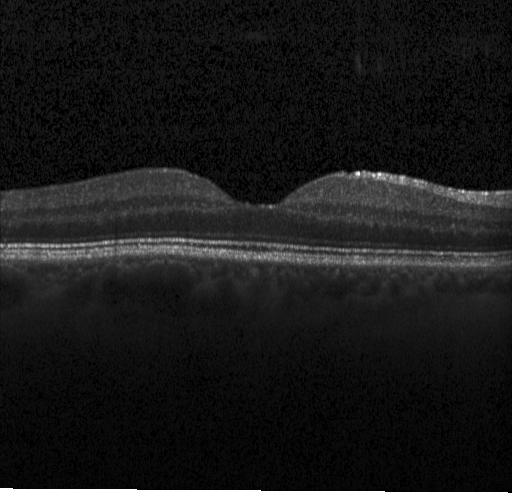 Spectral-domain optical coherence tomography · OCT B-scan
Impression: no choroidal neovascularization, diabetic macular edema, or drusen.